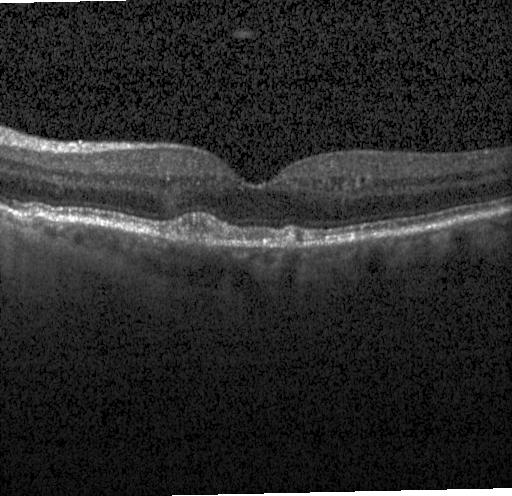

Heidelberg Spectralis. OCT B-scan. Centered on the fovea.
Assessment: drusen.